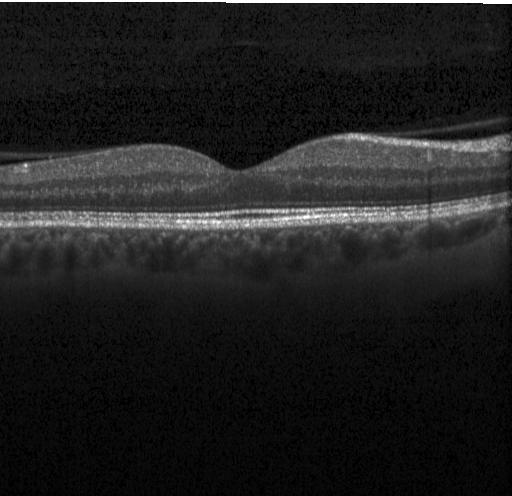 Optical coherence tomography scan
The scan shows no CNV, no DME, and no drusen.